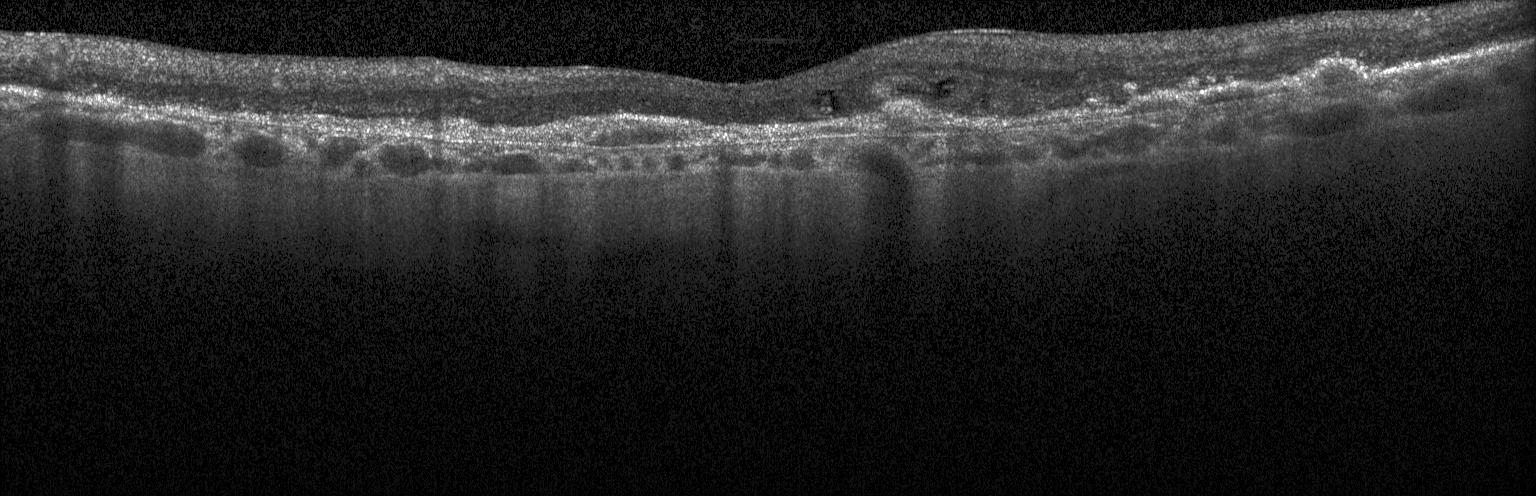

OCT B-scan showing a choroidal neovascular membrane.